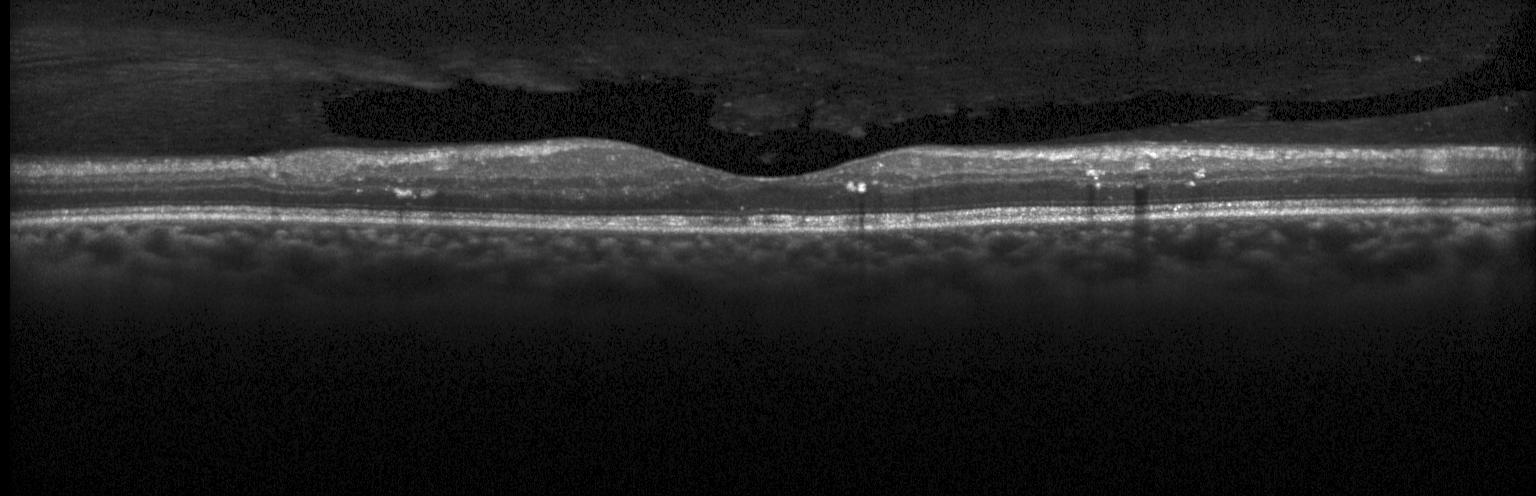 Finding: DME.